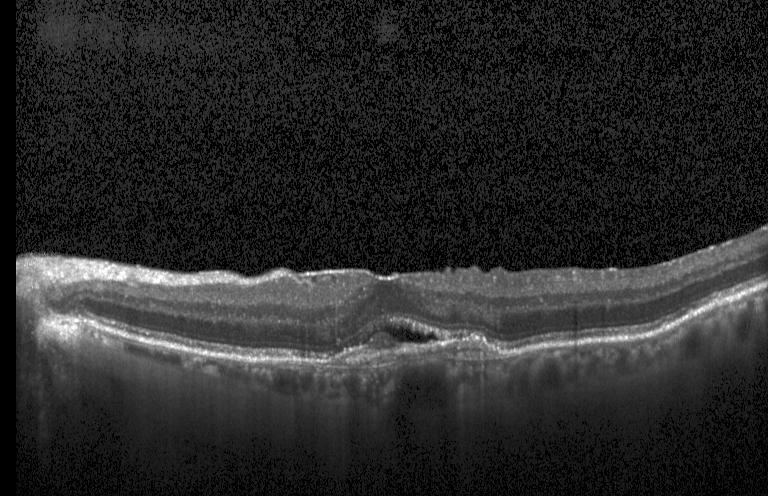
SD-OCT; optical coherence tomography B-scan
This B-scan demonstrates choroidal neovascularization.